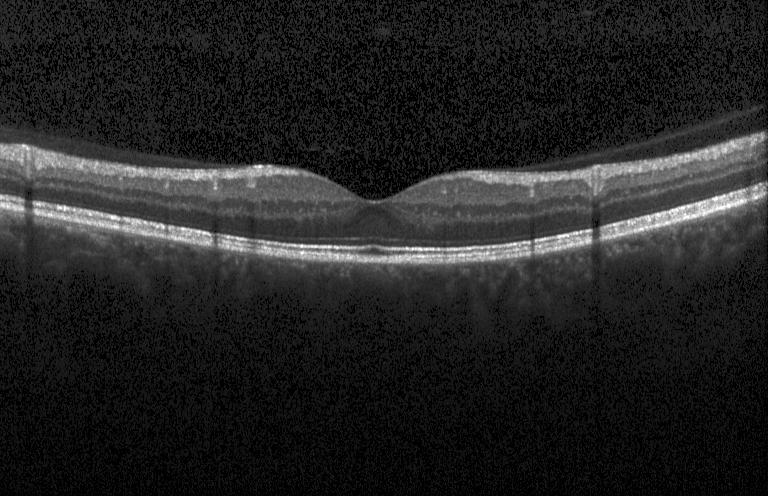 Through the macula; OCT B-scan
Macular OCT: neither CNV, DME, nor drusen.